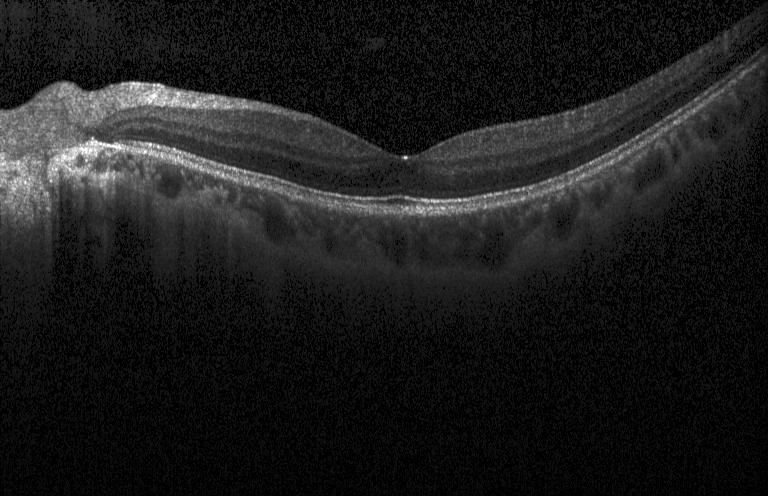

Optical coherence tomography B-scan — No CNV, DME, or drusen.